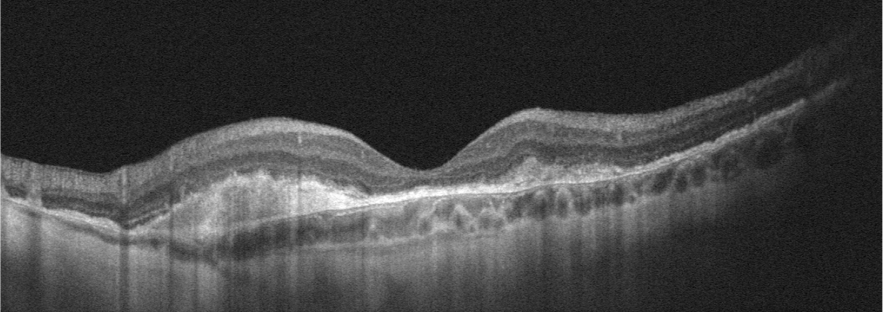
OCT finding: age-related macular degeneration (AMD).